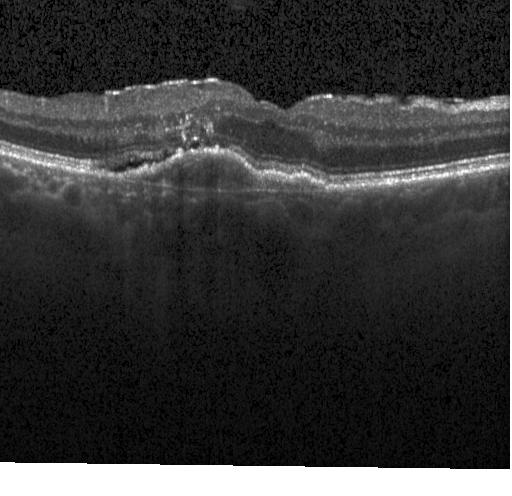

Retinal OCT B-scan, spectral-domain OCT
Impression: CNV.